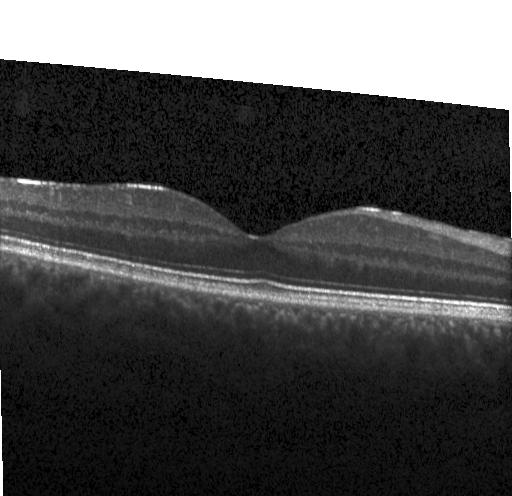
Retinal OCT cross-section
The scan shows no evidence of CNV, DME, or drusen.